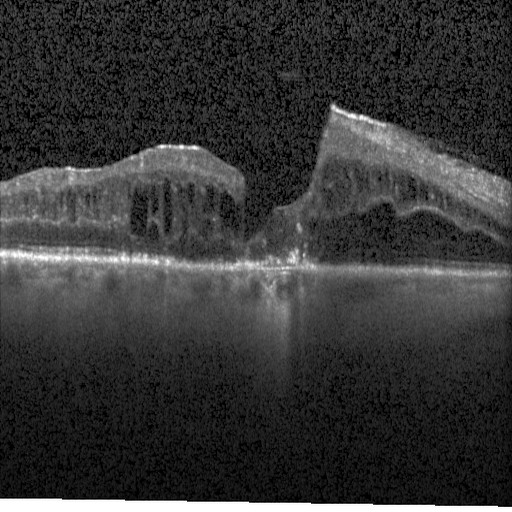
Instrument: Heidelberg Spectralis; fovea-centered; retinal OCT B-scan
Diagnosis: diabetic macular edema (DME).